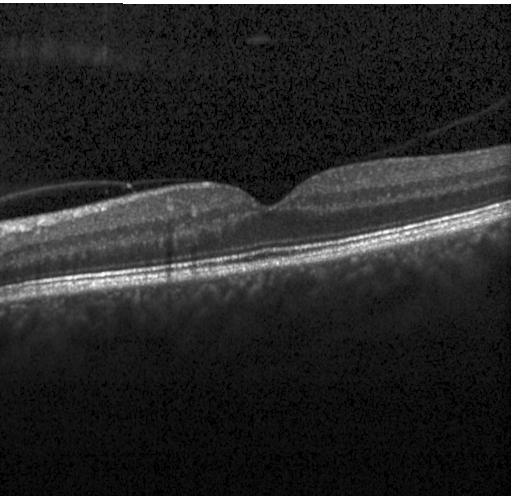

Fovea-centered · optical coherence tomography scan · spectral-domain optical coherence tomography — Finding: no choroidal neovascularization, diabetic macular edema, or drusen.